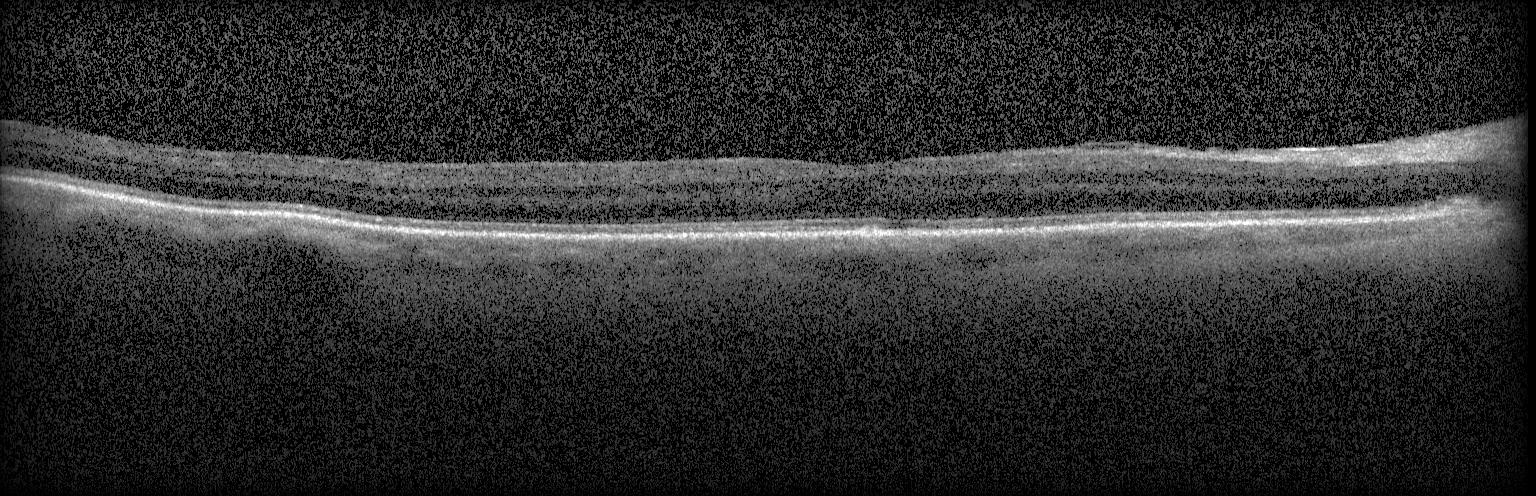
Diagnosis: no choroidal neovascularization, diabetic macular edema, or drusen.